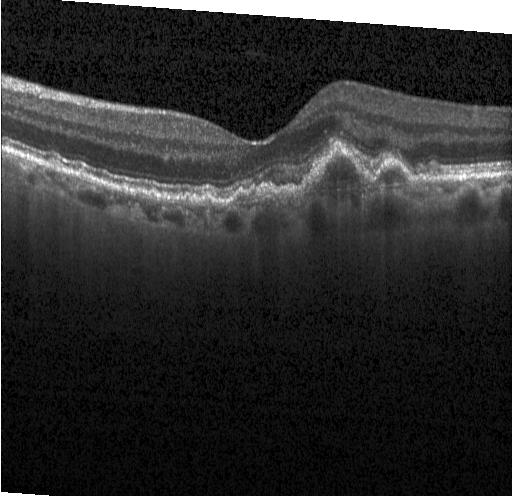 Instrument: Heidelberg Spectralis, retinal OCT cross-section, SD-OCT, macular scan.
OCT finding: choroidal neovascularization (CNV).